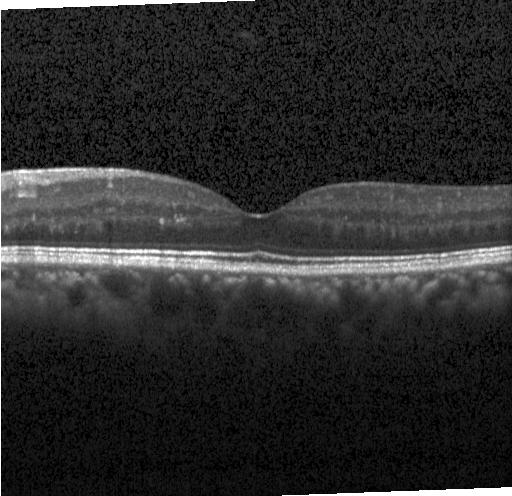 Retinal OCT cross-section showing neither CNV, DME, nor drusen.